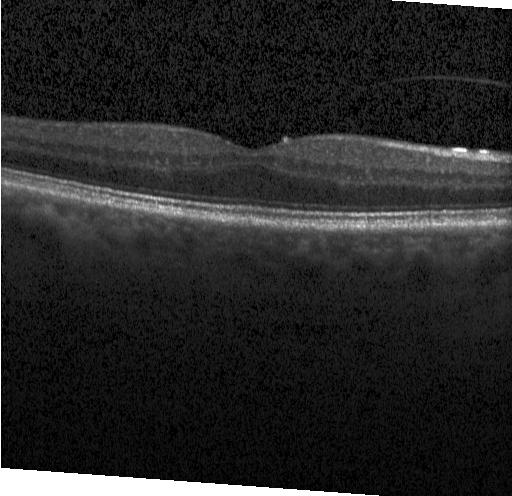

Spectral-domain OCT, fovea-centered, OCT B-scan
This B-scan demonstrates no CNV, DME, or drusen.